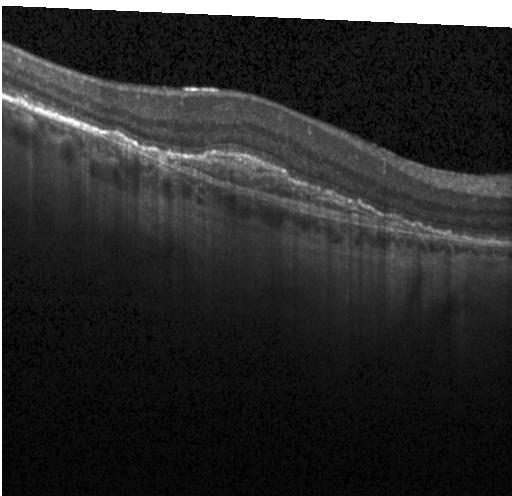

OCT B-scan showing choroidal neovascularization (CNV).